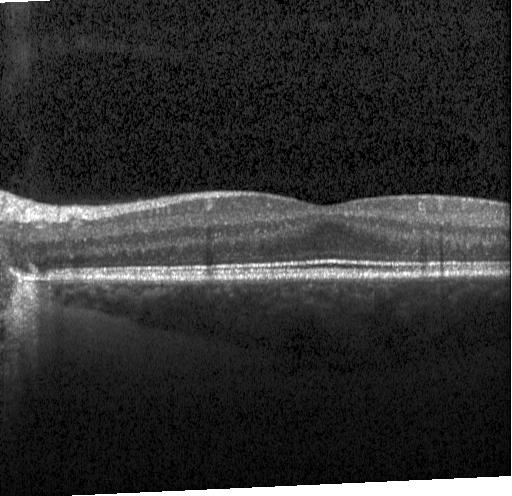 OCT line scan — This B-scan demonstrates neither choroidal neovascularization, diabetic macular edema, nor drusen.